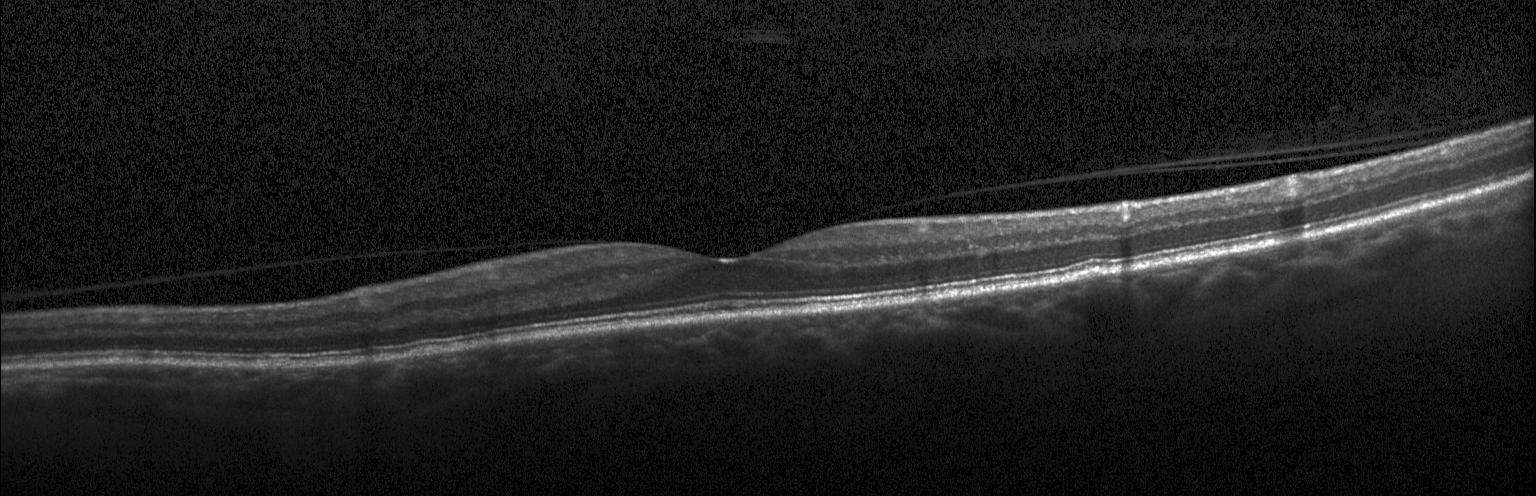 OCT B-scan showing no choroidal neovascularization, no diabetic macular edema, and no drusen.